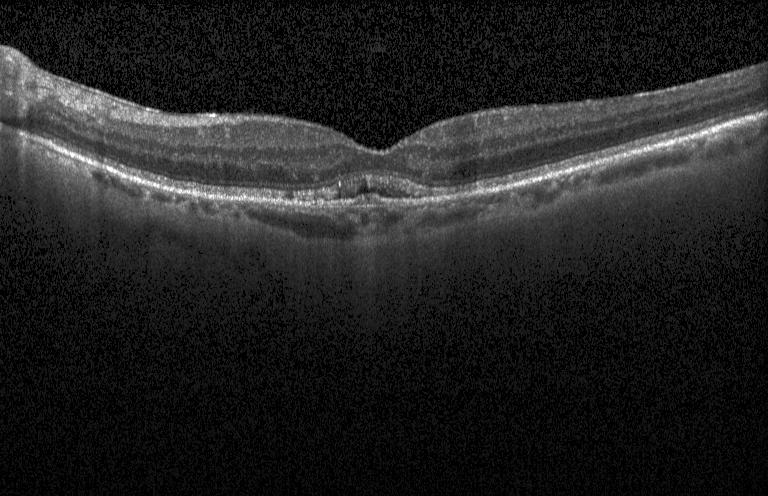 OCT line scan. A choroidal neovascular membrane.